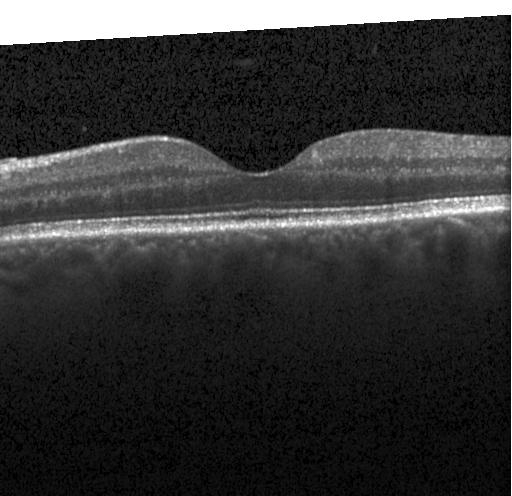

Optical coherence tomography scan; centered on the fovea.
Diagnosis: no choroidal neovascularization, diabetic macular edema, or drusen.